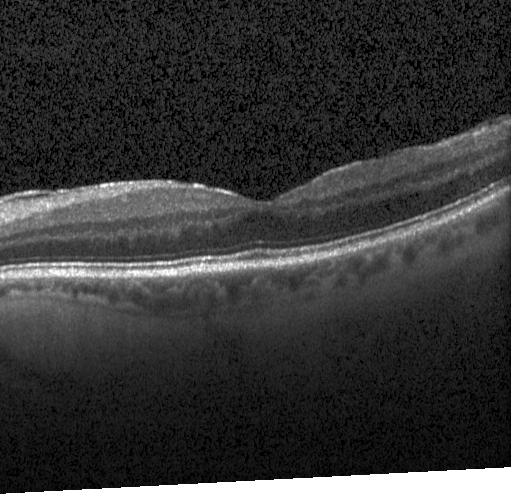
Optical coherence tomography B-scan · acquired on a Heidelberg Spectralis · through the macula
The scan shows no CNV, no DME, and no drusen.